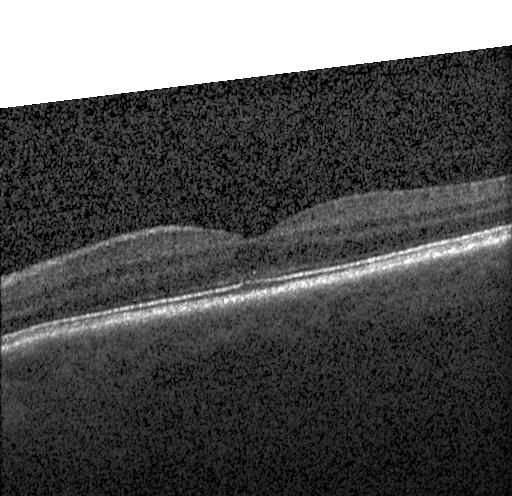

SD-OCT. Retinal OCT B-scan. Fovea-centered.
Diagnosis: neither CNV, DME, nor drusen.